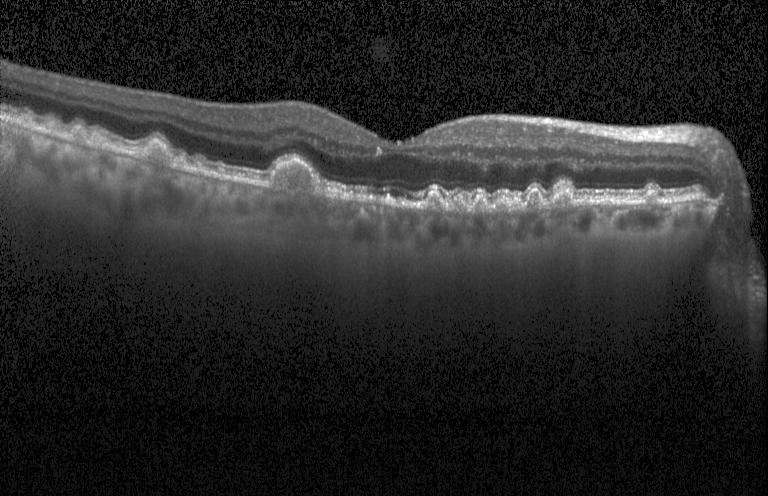

Diagnosis: drusen.